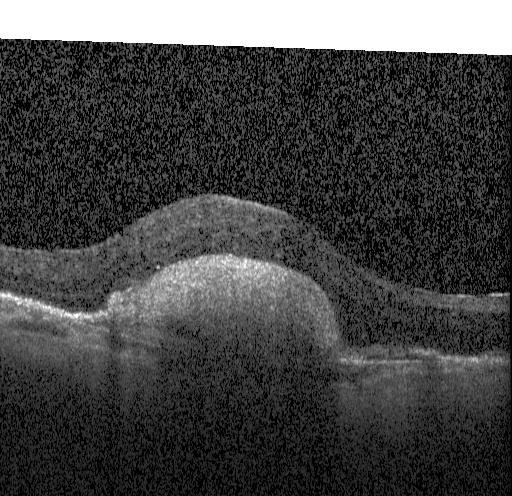
Retinal OCT cross-section
The scan shows choroidal neovascularization.